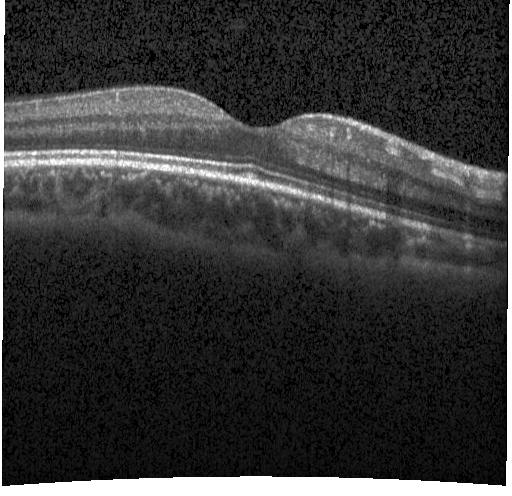 Macular scan, spectral-domain OCT, OCT line scan.
Assessment: no choroidal neovascularization, diabetic macular edema, or drusen.